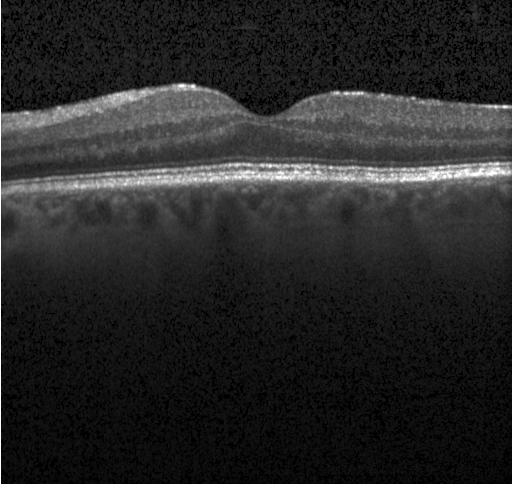 OCT finding: neither choroidal neovascularization, diabetic macular edema, nor drusen.